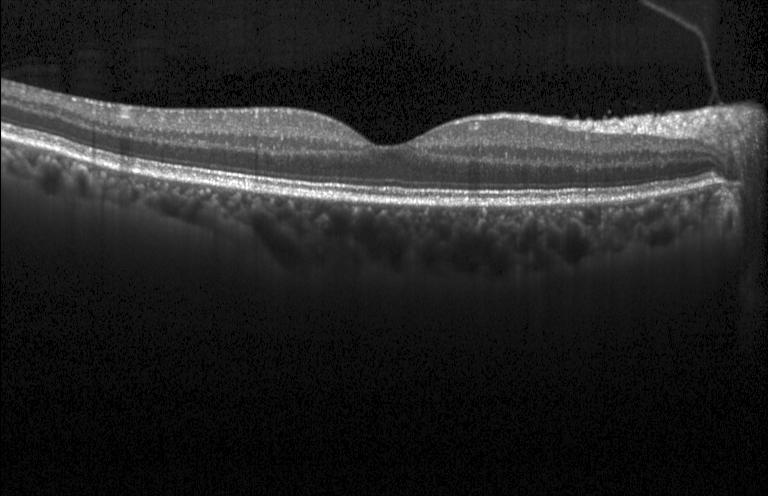

Spectral-domain OCT · instrument: Heidelberg Spectralis · centered on the fovea · retinal OCT cross-section.
Impression: no CNV, no DME, and no drusen.